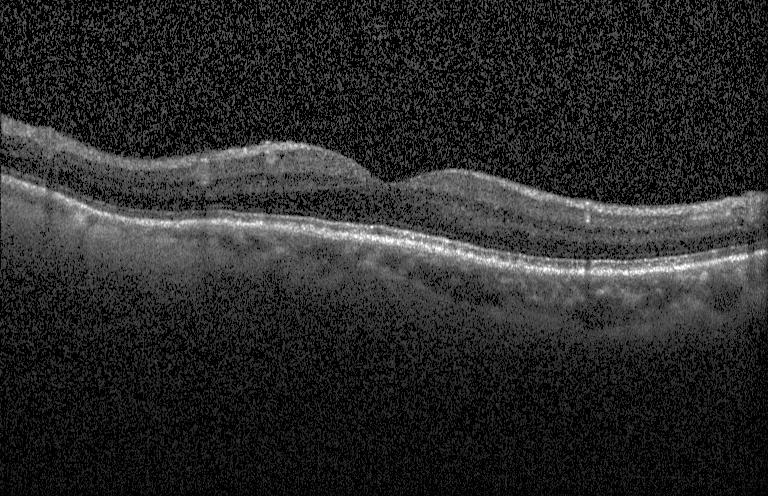

Spectral-domain OCT, optical coherence tomography scan. Impression: no choroidal neovascularization, diabetic macular edema, or drusen.